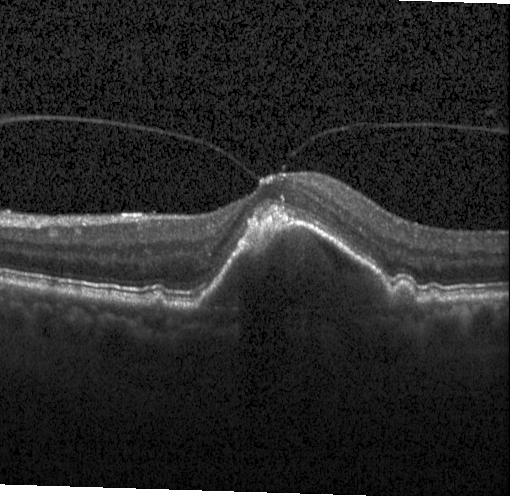 Dx: CNV.